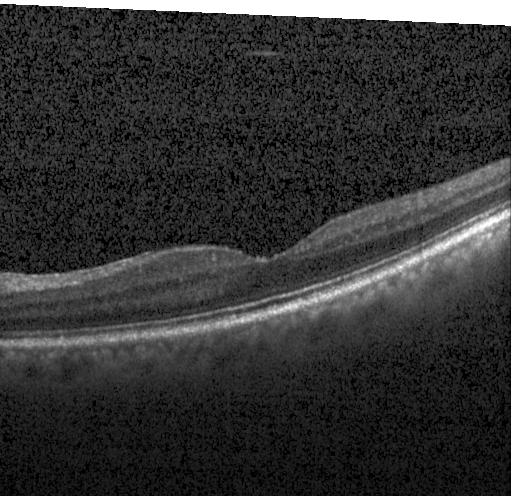 OCT B-scan showing no evidence of choroidal neovascularization, diabetic macular edema, or drusen.